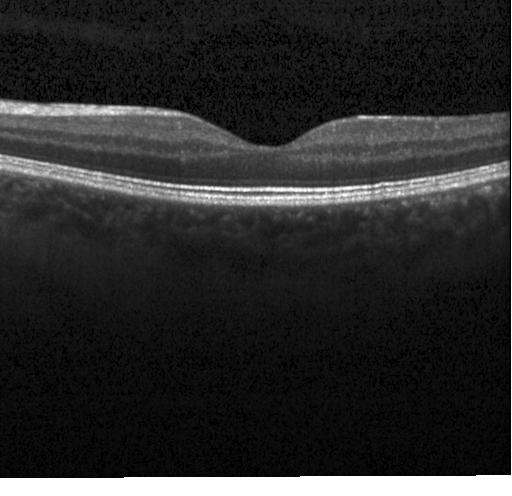 OCT line scan
Finding: no CNV, DME, or drusen.